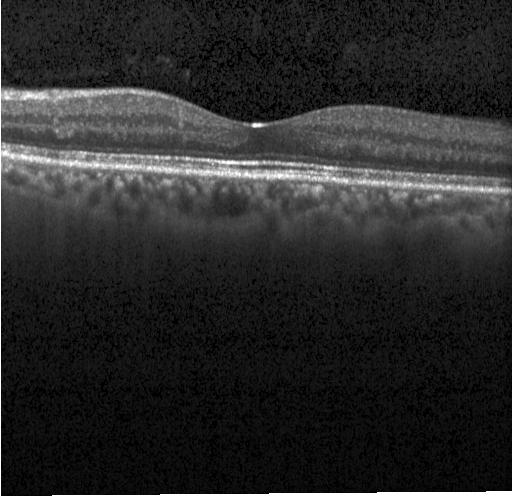
Dx: no choroidal neovascularization, diabetic macular edema, or drusen.